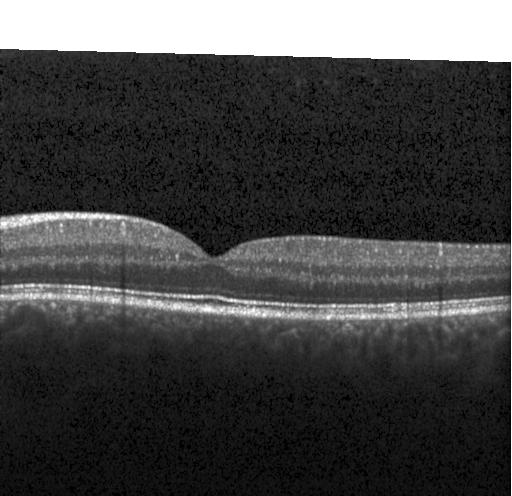

Fovea-centered · SD-OCT · retinal OCT cross-section · acquired on a Heidelberg Spectralis — Dx: no choroidal neovascularization, no diabetic macular edema, and no drusen.